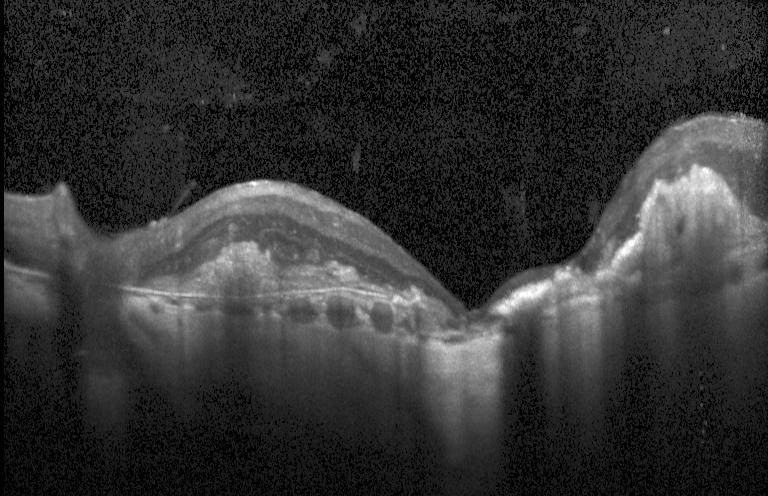
Assessment: a choroidal neovascular membrane.